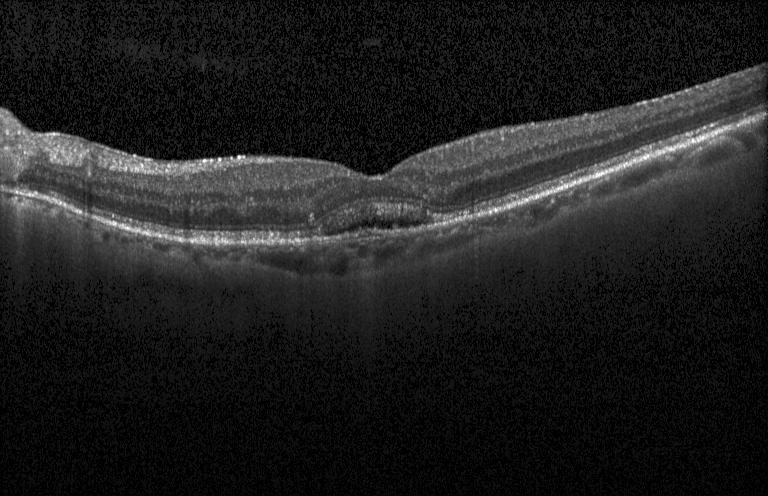 Spectral-domain optical coherence tomography, optical coherence tomography B-scan, horizontal scan through the fovea.
Finding: CNV.